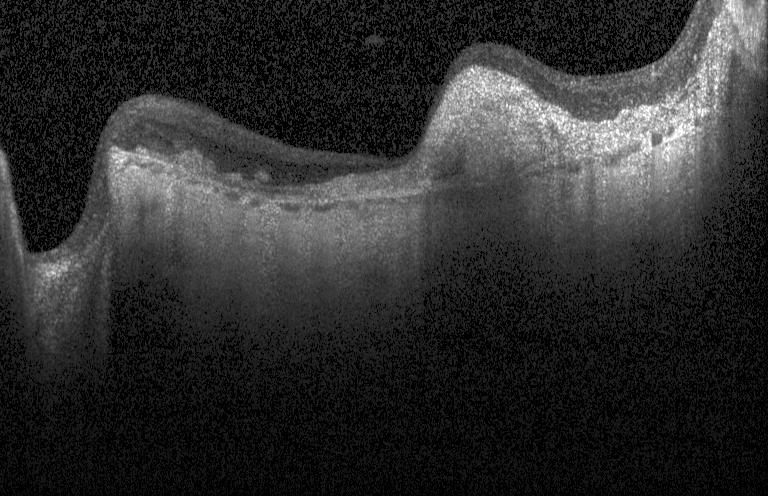
Diagnosis: a choroidal neovascular membrane.